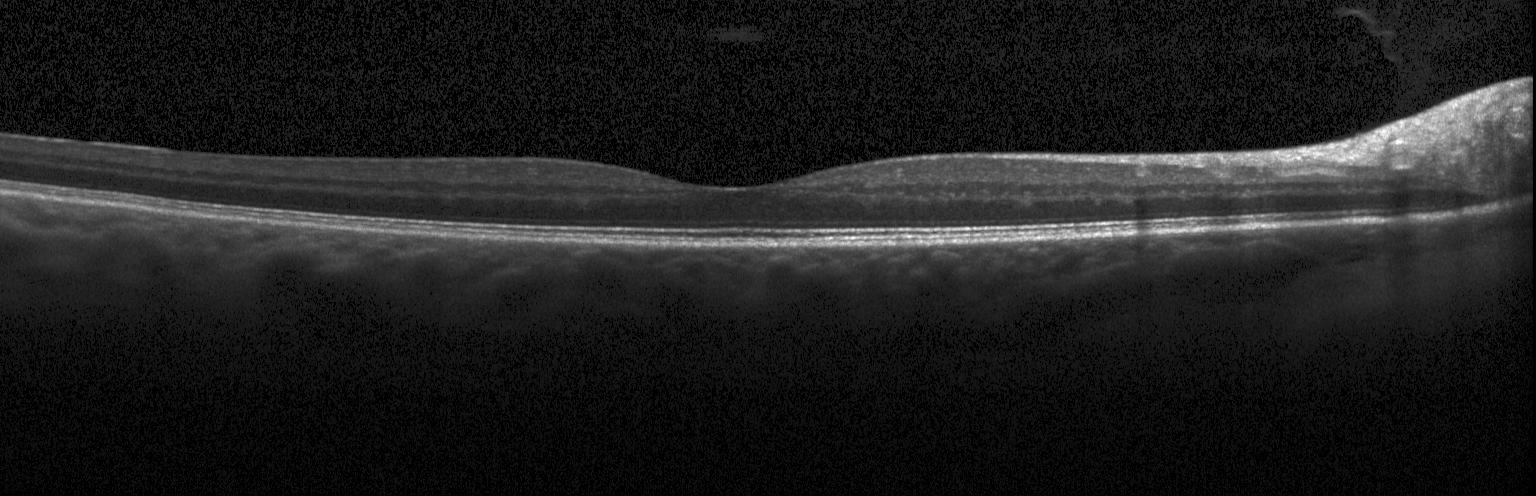 Impression: no choroidal neovascularization, no diabetic macular edema, and no drusen.